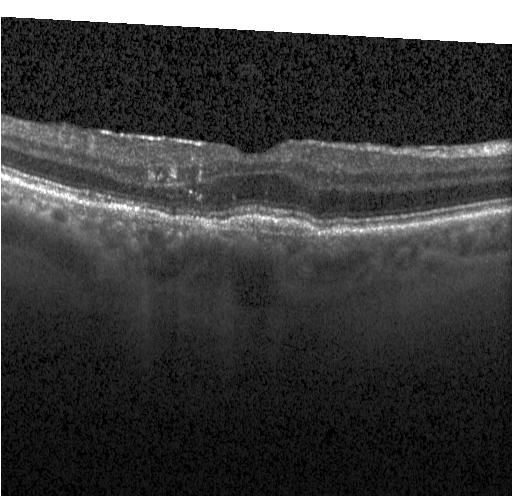 Macular scan, SD-OCT, optical coherence tomography scan, instrument: Heidelberg Spectralis.
Assessment: choroidal neovascularization.